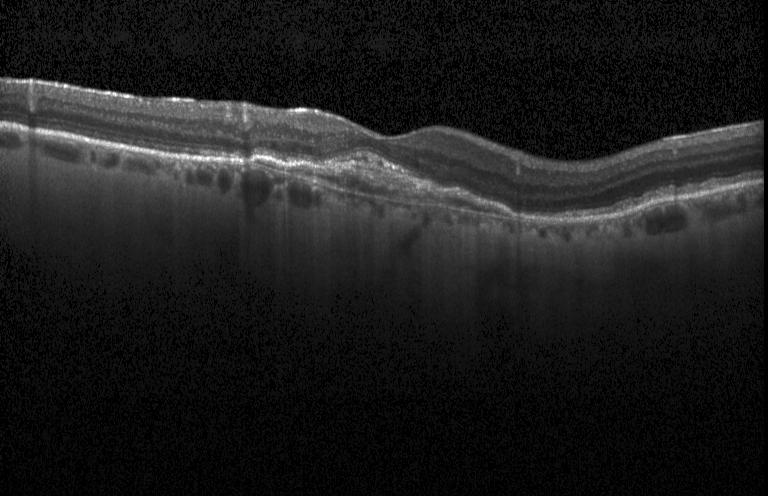 Fovea-centered, instrument: Heidelberg Spectralis, optical coherence tomography B-scan
OCT finding: a choroidal neovascular membrane.